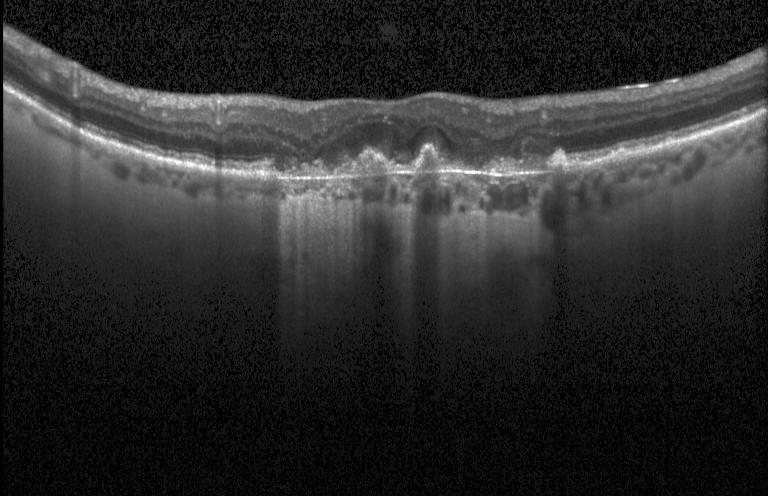 Fovea-centered. OCT line scan — OCT finding: choroidal neovascularization.